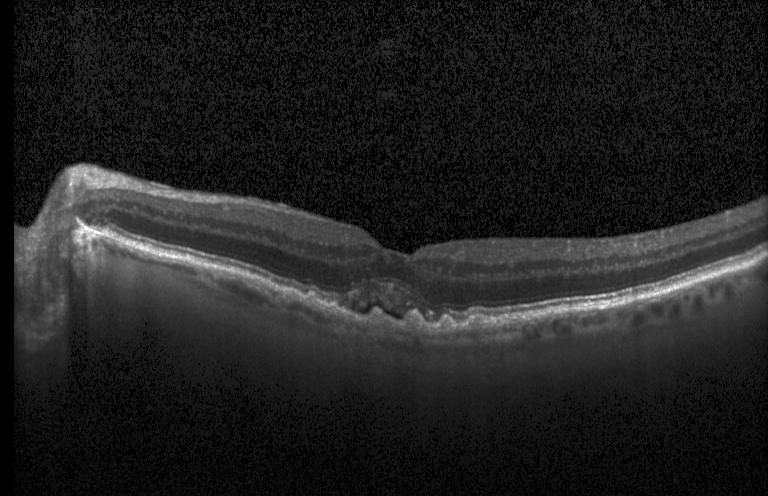
Optical coherence tomography B-scan · macular scan · spectral-domain optical coherence tomography — A choroidal neovascular membrane.